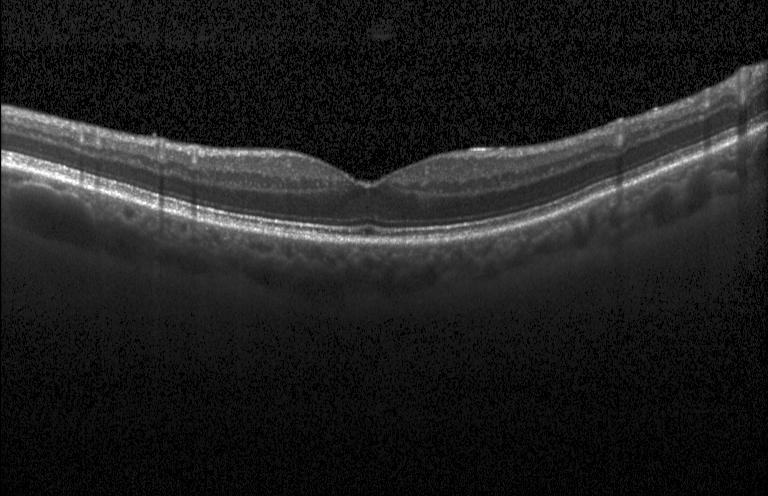 Fovea-centered. Acquired on a Heidelberg Spectralis. SD-OCT. Retinal OCT B-scan — Finding: no choroidal neovascularization, diabetic macular edema, or drusen.